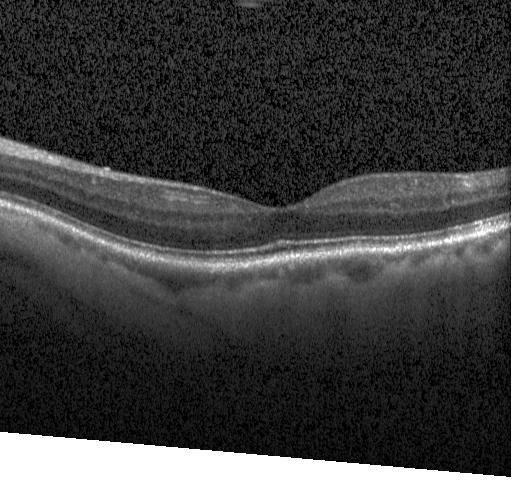

Macular OCT demonstrating no CNV, DME, or drusen.